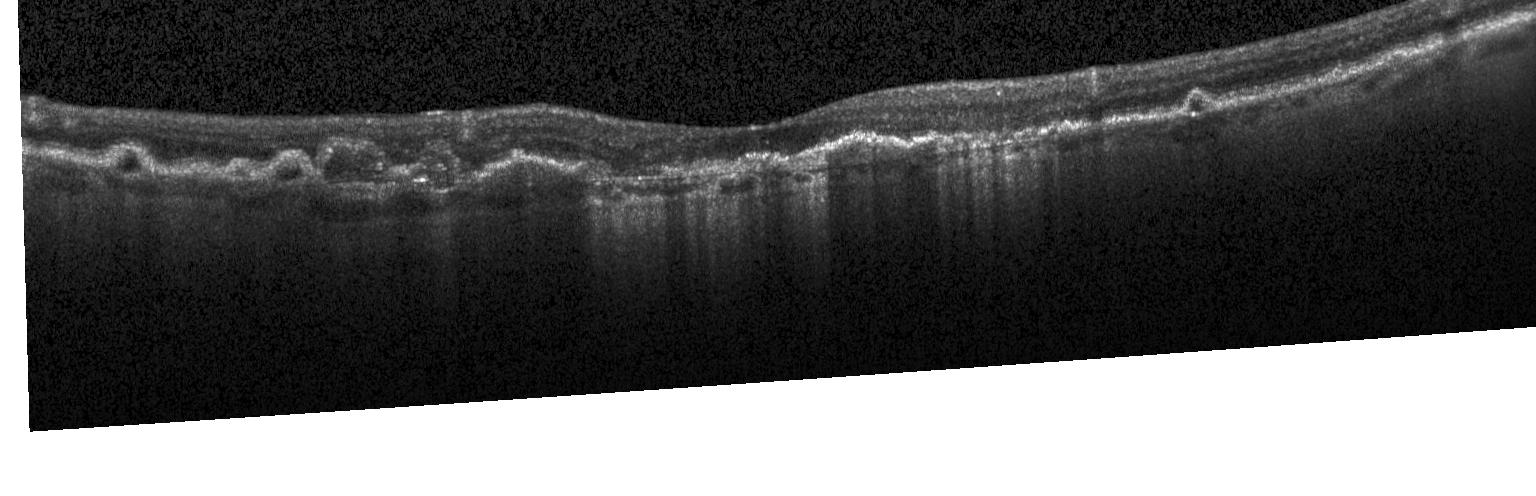 Retinal OCT cross-section · macular scan
Impression: CNV.